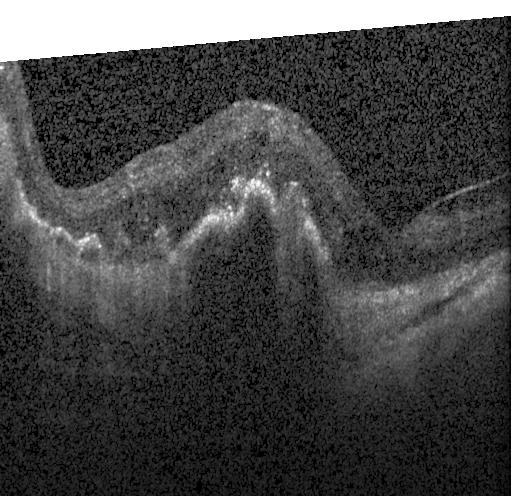

Spectral-domain optical coherence tomography · horizontal scan through the fovea · Heidelberg Spectralis · retinal OCT B-scan. Finding: a choroidal neovascular membrane.